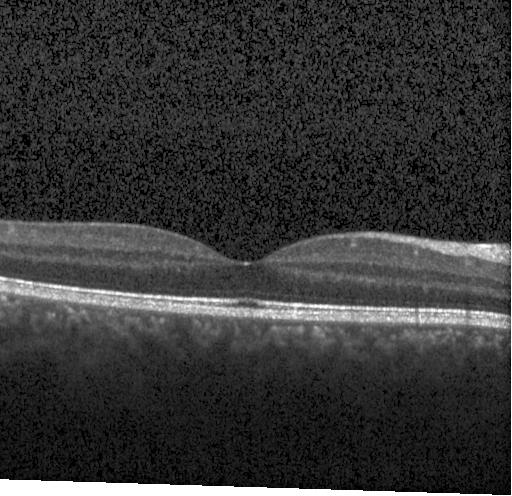

OCT line scan · Heidelberg Spectralis OCT system · horizontal scan through the fovea.
No evidence of choroidal neovascularization, diabetic macular edema, or drusen.